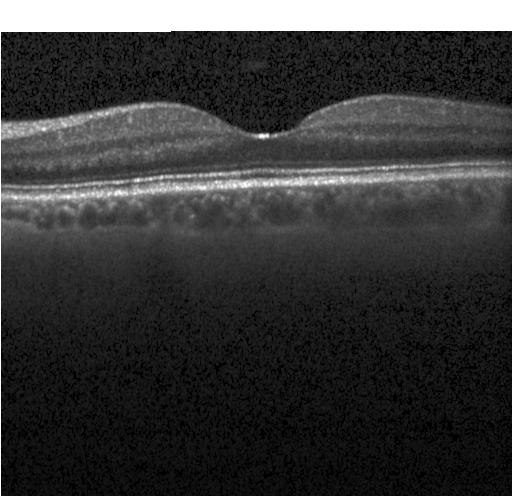

Neither choroidal neovascularization, diabetic macular edema, nor drusen.